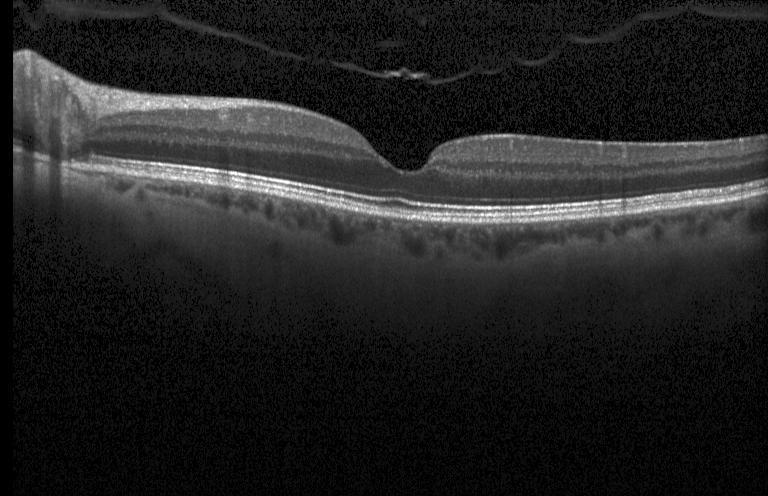 This B-scan demonstrates neither choroidal neovascularization, diabetic macular edema, nor drusen.